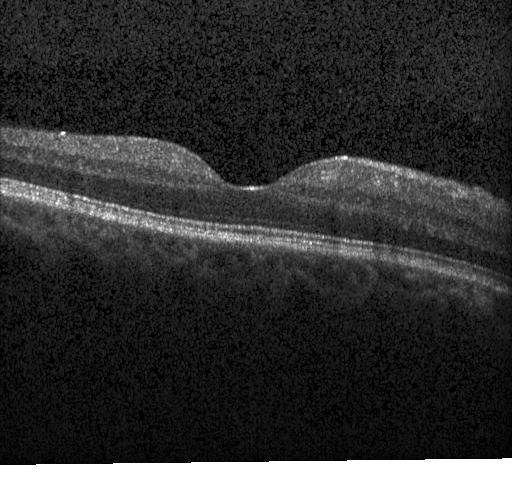
Retinal OCT B-scan — OCT finding: no CNV, no DME, and no drusen.